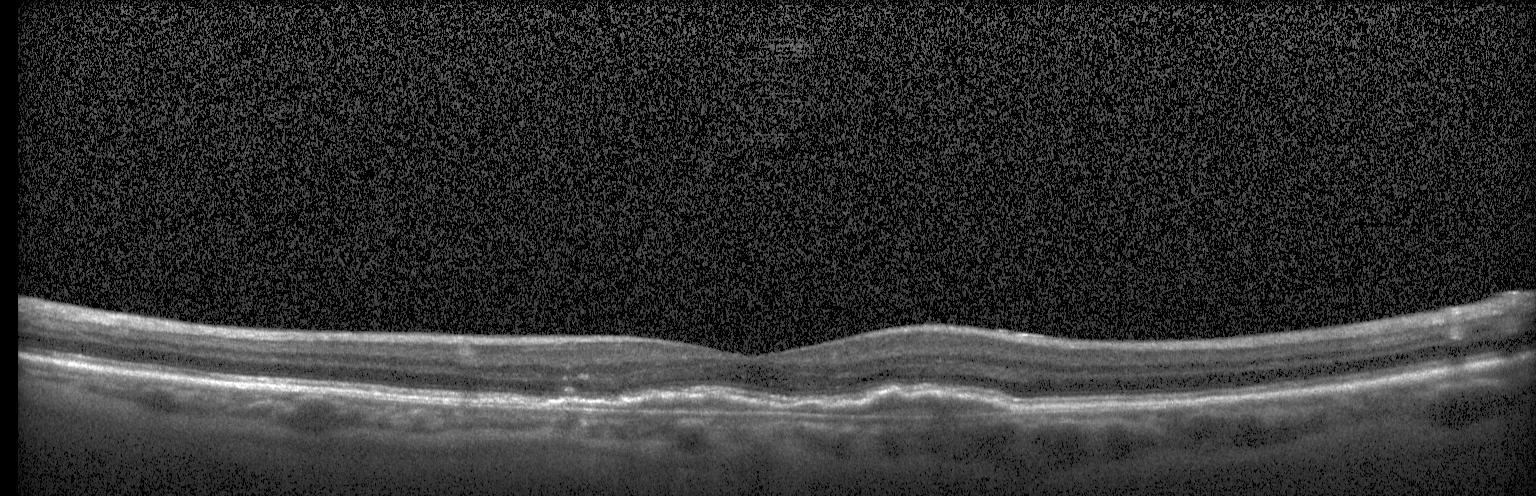 Optical coherence tomography scan · through the macula · Heidelberg Spectralis OCT system — Diagnosis: a choroidal neovascular membrane.